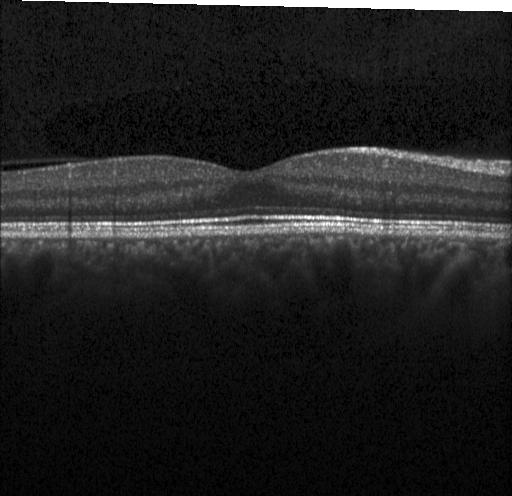
Finding: no evidence of choroidal neovascularization, diabetic macular edema, or drusen.